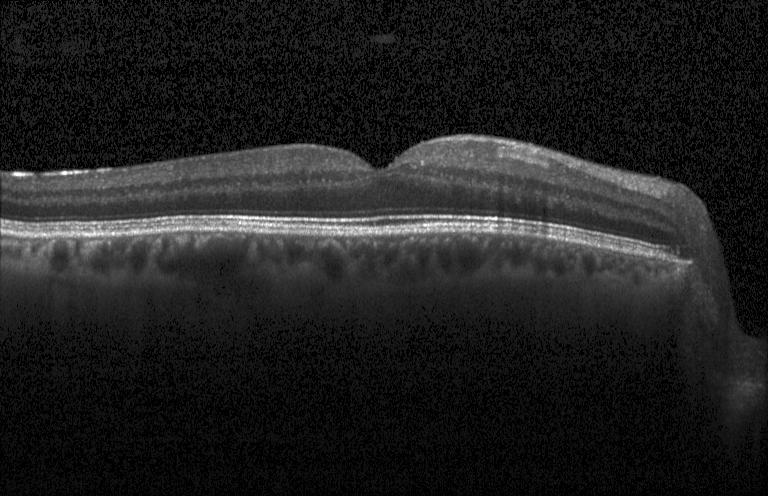
OCT B-scan showing no evidence of CNV, DME, or drusen.